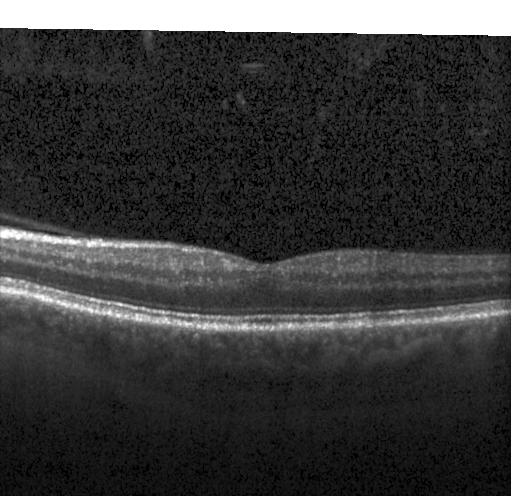
Optical coherence tomography B-scan. Diagnosis: no choroidal neovascularization, diabetic macular edema, or drusen.